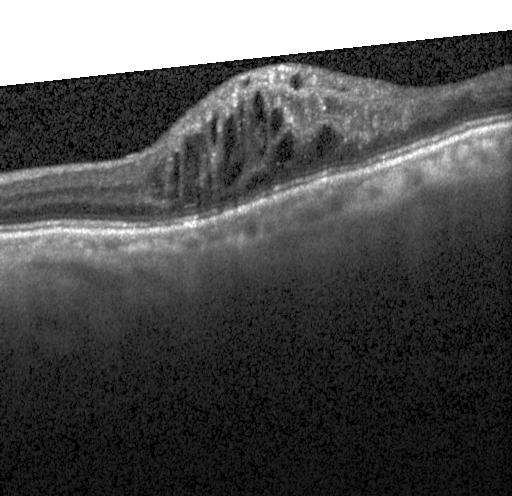
Macular OCT demonstrating diabetic macular edema.